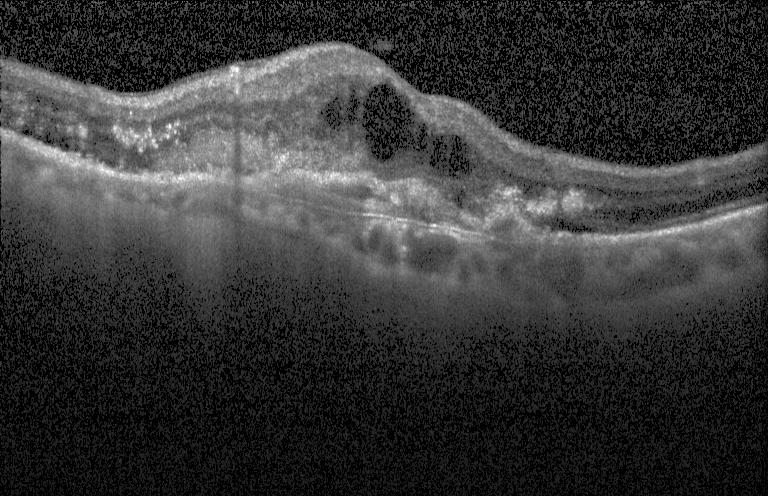

OCT scan showing a choroidal neovascular membrane.